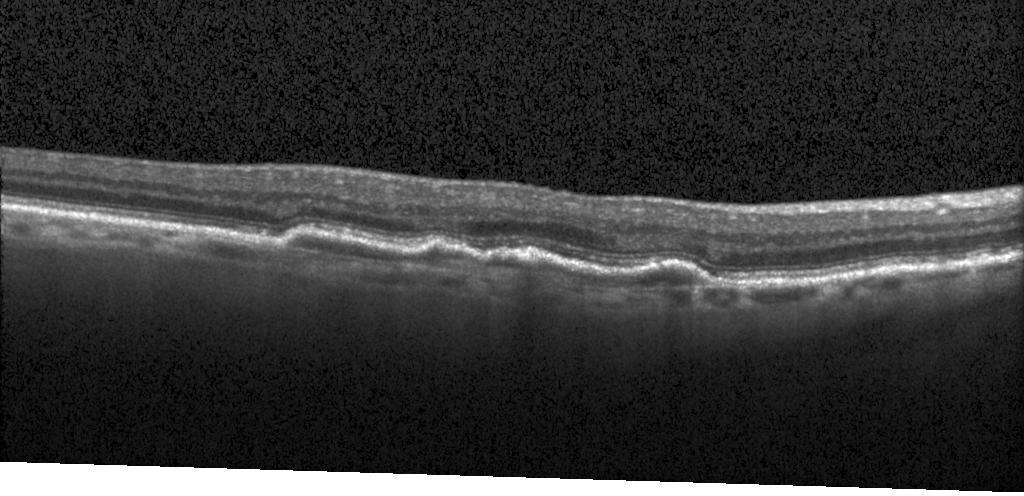 Macular OCT: CNV.